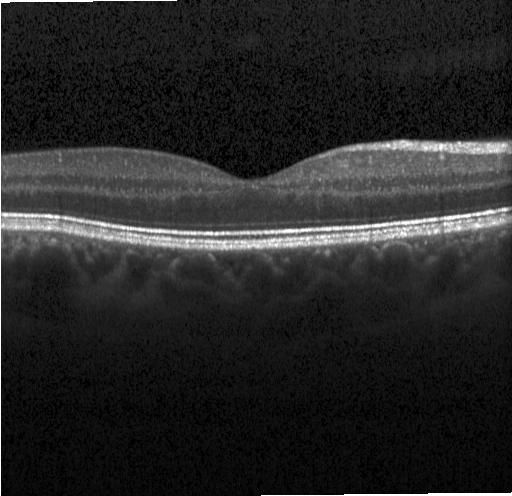

Retinal OCT cross-section. Spectral-domain optical coherence tomography — Macular OCT: no CNV, no DME, and no drusen.